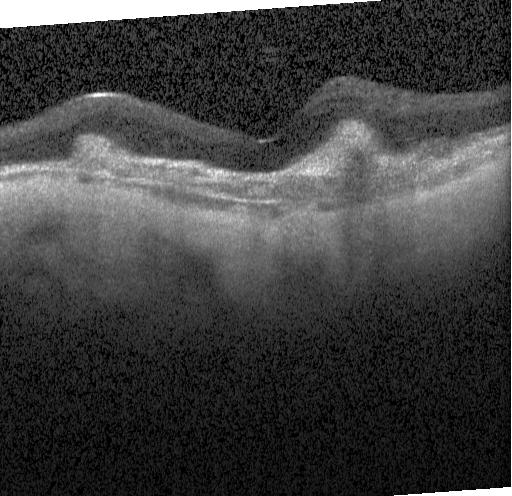 Impression: choroidal neovascularization.